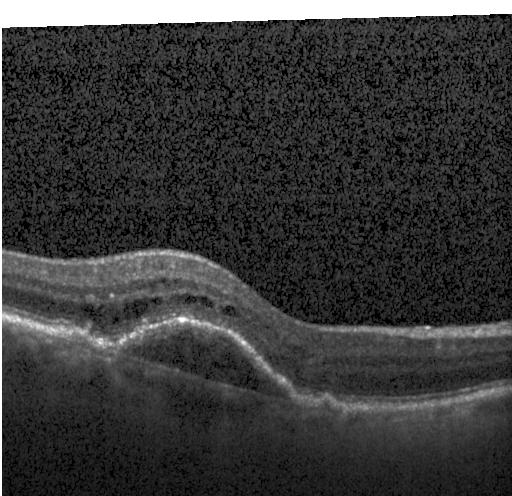 Dx: CNV.